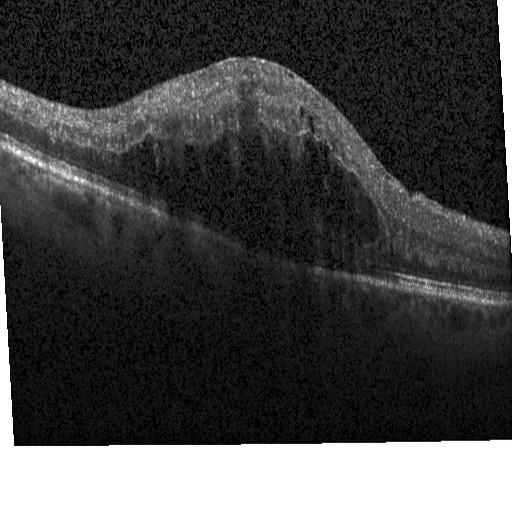
Instrument: Heidelberg Spectralis; retinal OCT B-scan; spectral-domain optical coherence tomography — Impression: diabetic macular edema.